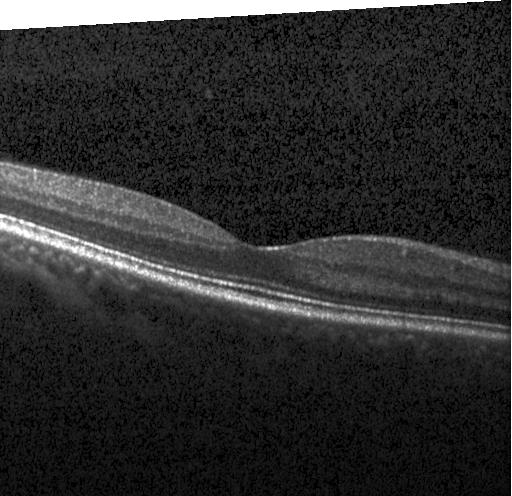
Optical coherence tomography scan; spectral-domain optical coherence tomography; macular scan
Macular OCT: no evidence of CNV, DME, or drusen.